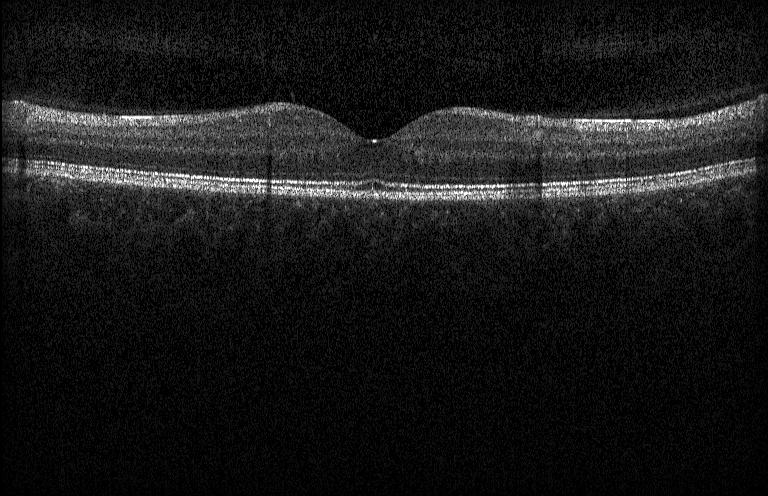
Optical coherence tomography scan.
Finding: no evidence of CNV, DME, or drusen.